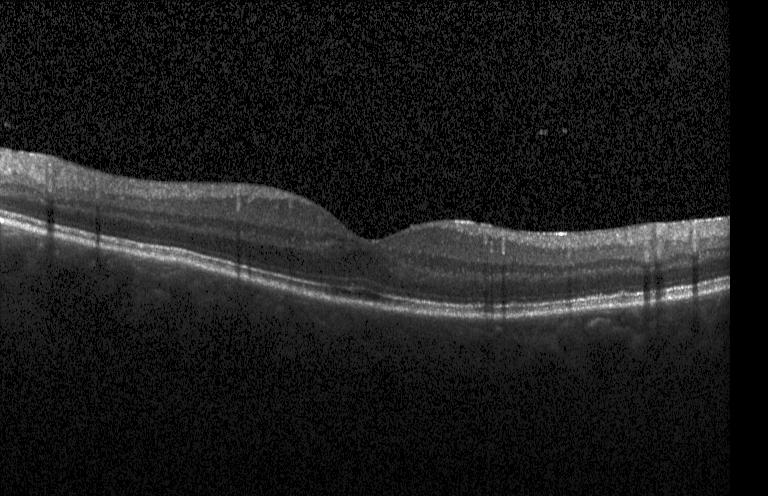 Macular OCT: neither choroidal neovascularization, diabetic macular edema, nor drusen.